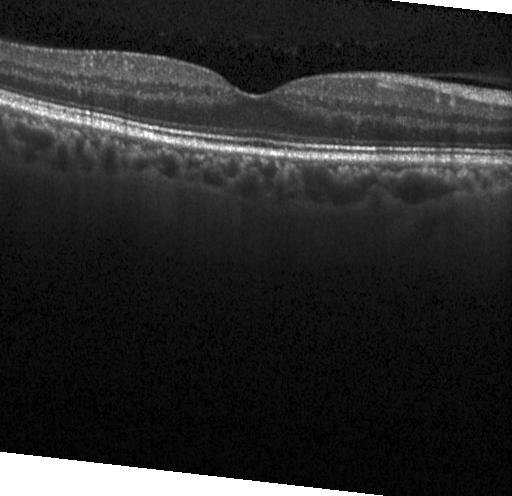 Diagnosis: neither choroidal neovascularization, diabetic macular edema, nor drusen.